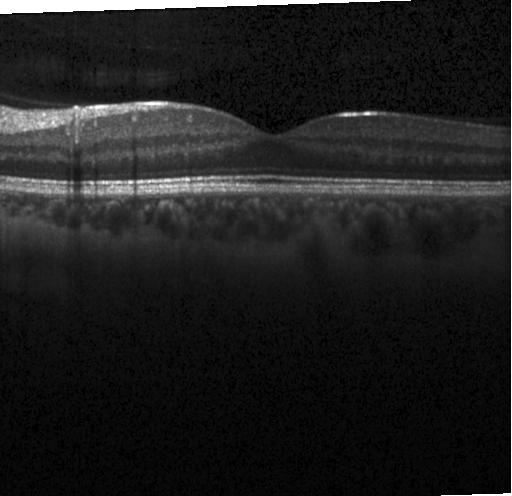

Impression: neither choroidal neovascularization, diabetic macular edema, nor drusen.